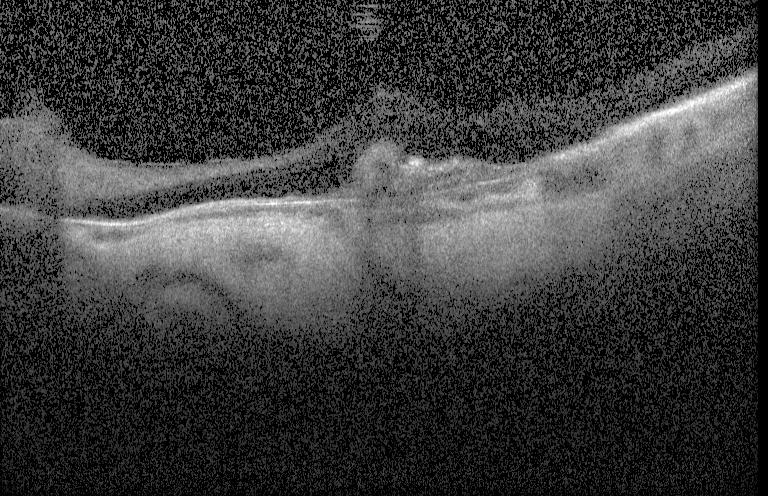

Retinal OCT cross-section. A choroidal neovascular membrane.